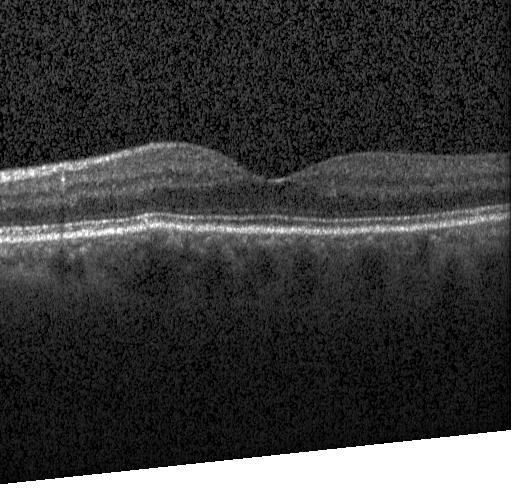

OCT line scan.
OCT finding: no choroidal neovascularization, diabetic macular edema, or drusen.